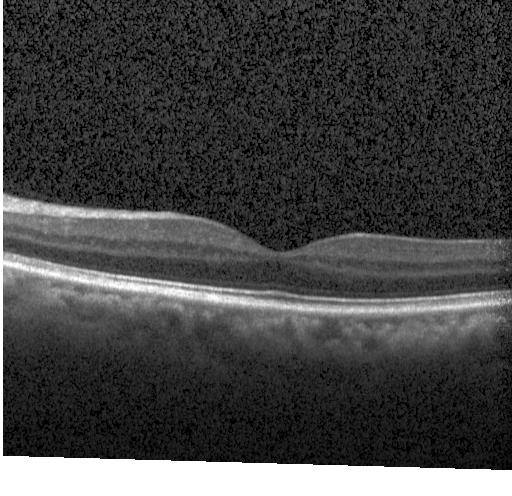

Retinal OCT B-scan. Diagnosis: no choroidal neovascularization, no diabetic macular edema, and no drusen.